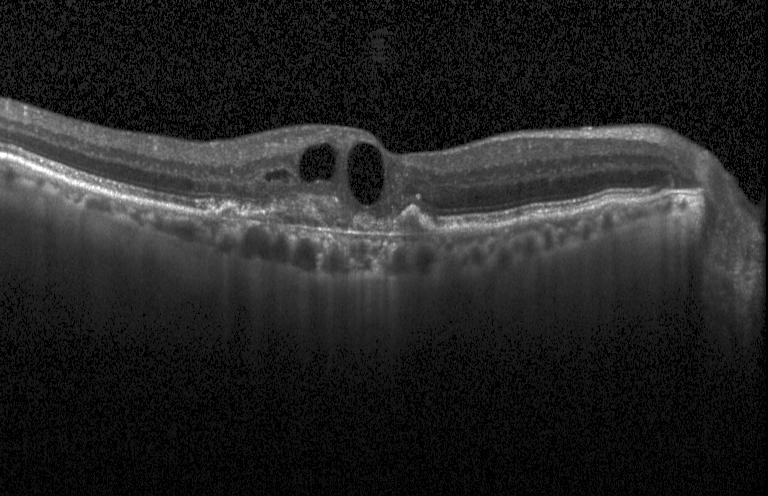

Retinal OCT cross-section · fovea-centered
Diagnosis: a choroidal neovascular membrane.